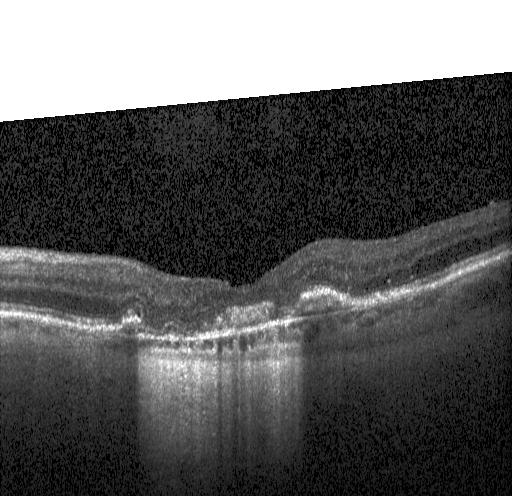

SD-OCT · optical coherence tomography B-scan · acquired on a Heidelberg Spectralis
Diagnosis: CNV.